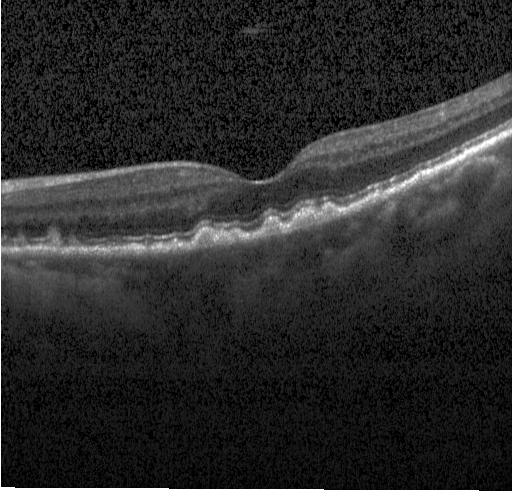
OCT B-scan. Spectral-domain OCT. Heidelberg Spectralis OCT system.
Assessment: drusen.